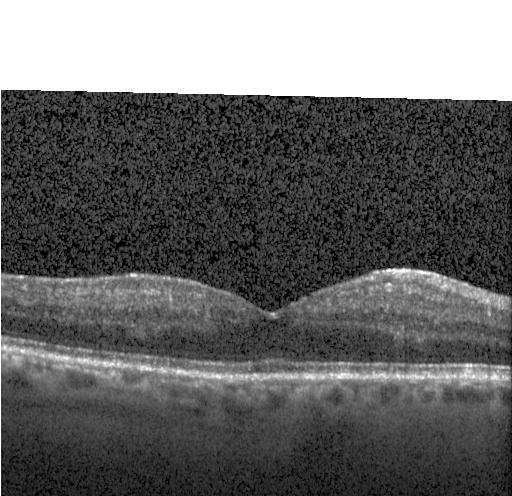
OCT B-scan, Heidelberg Spectralis OCT system, horizontal scan through the fovea. Impression: no choroidal neovascularization, no diabetic macular edema, and no drusen.